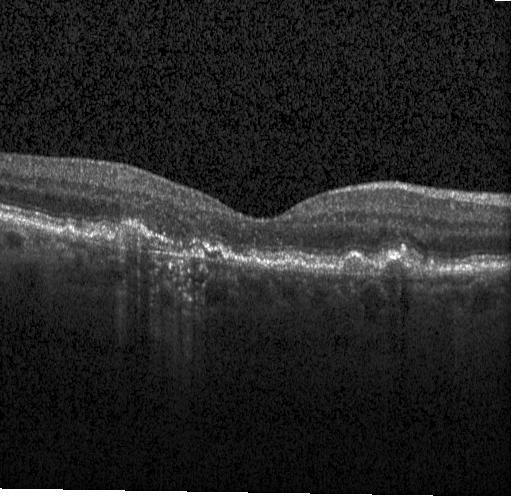
OCT finding: a choroidal neovascular membrane.